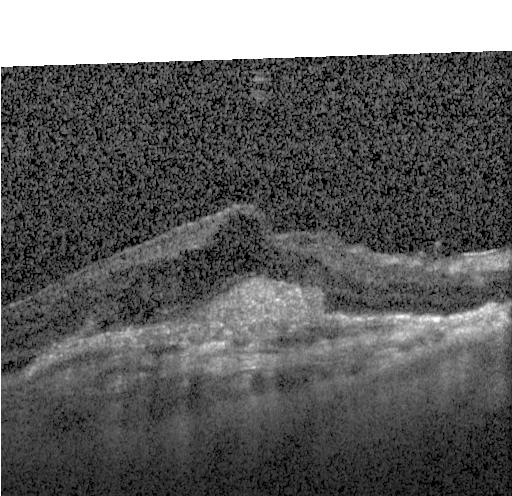
Retinal OCT cross-section · spectral-domain optical coherence tomography · Heidelberg Spectralis. Choroidal neovascularization (CNV).